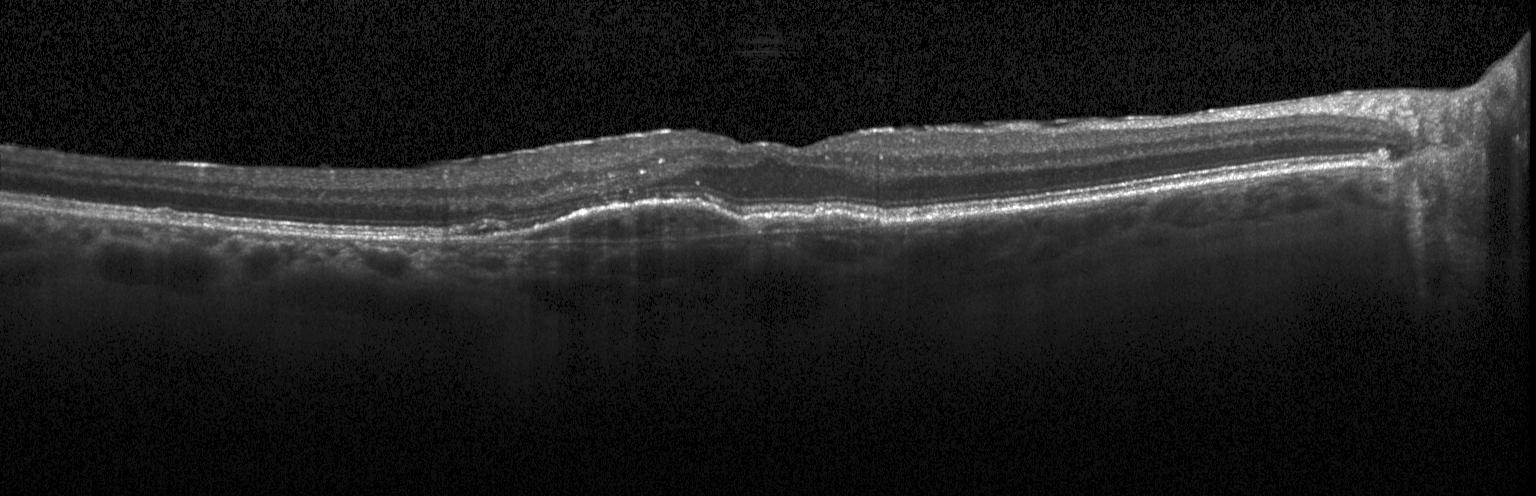

OCT finding: choroidal neovascularization (CNV).